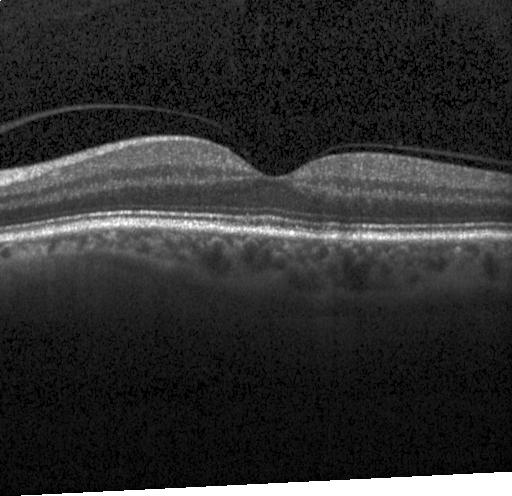

Retinal OCT cross-section
Diagnosis: no evidence of CNV, DME, or drusen.